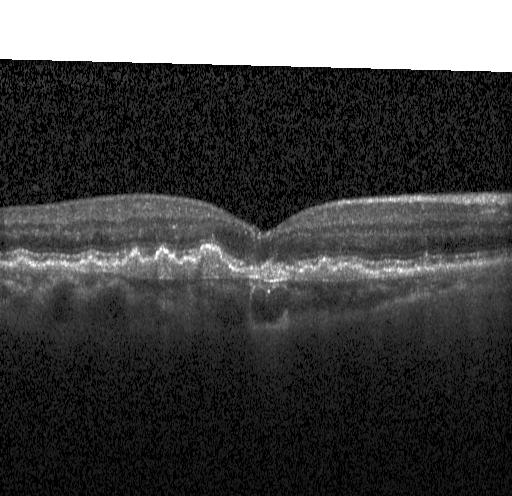

Assessment: a choroidal neovascular membrane.